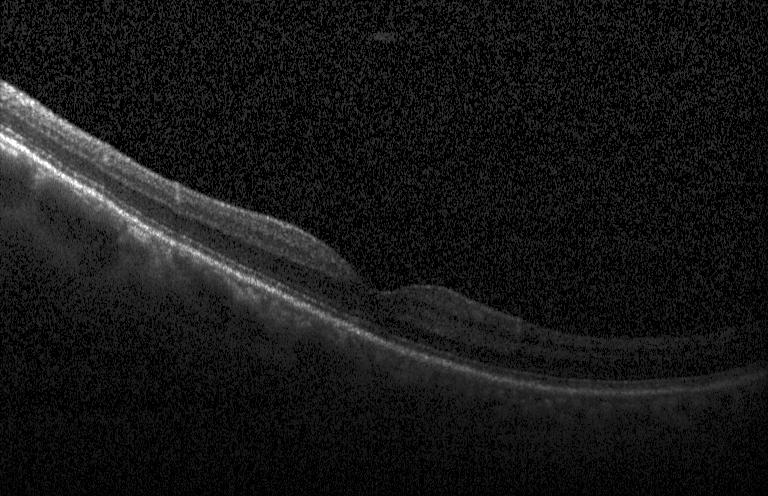

Spectral-domain OCT B-scan: no evidence of CNV, DME, or drusen.